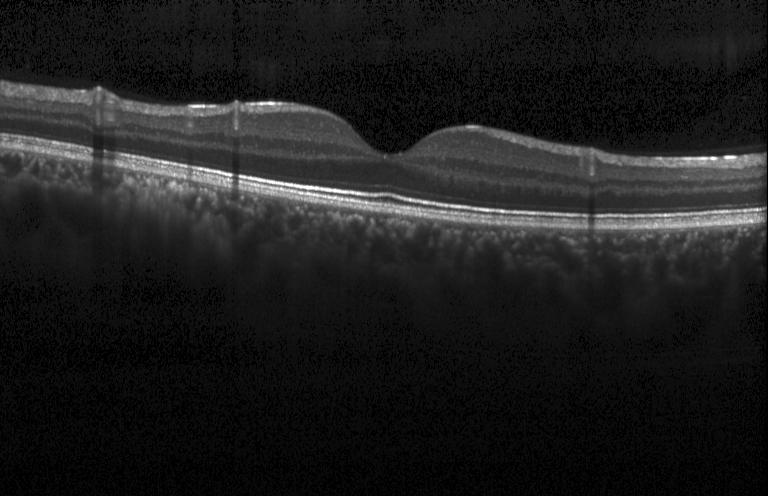 OCT line scan
The scan shows no CNV, no DME, and no drusen.